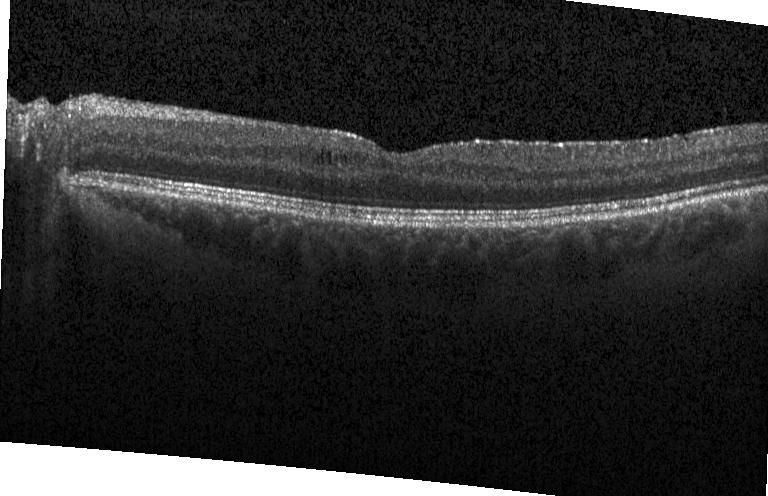 Finding: diabetic macular edema (DME).